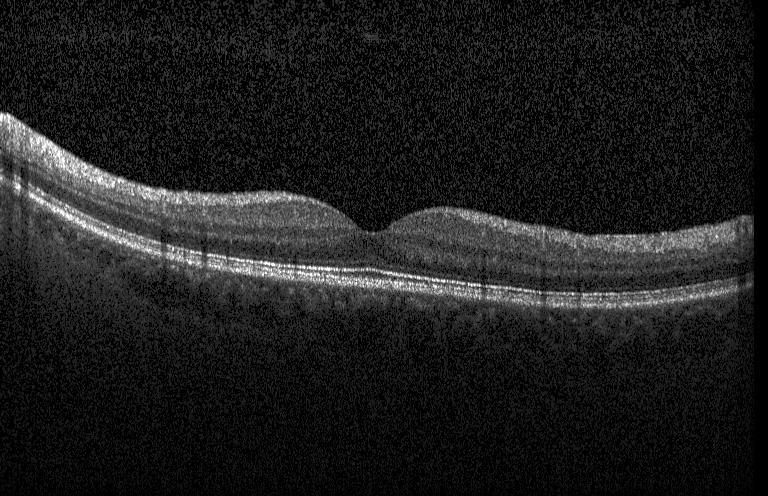
Macular scan · SD-OCT · optical coherence tomography scan · Heidelberg Spectralis — Finding: no evidence of choroidal neovascularization, diabetic macular edema, or drusen.